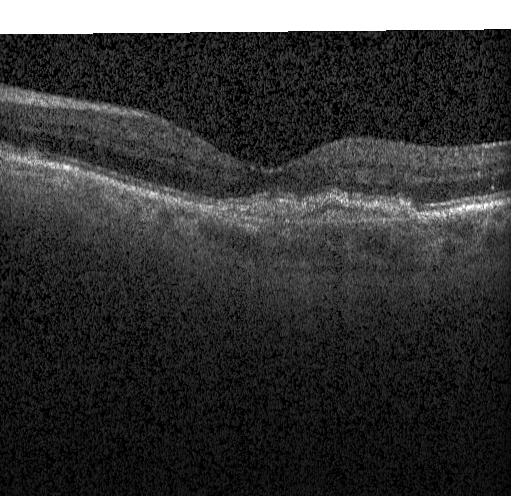
Optical coherence tomography B-scan; horizontal scan through the fovea.
Macular OCT: a choroidal neovascular membrane.